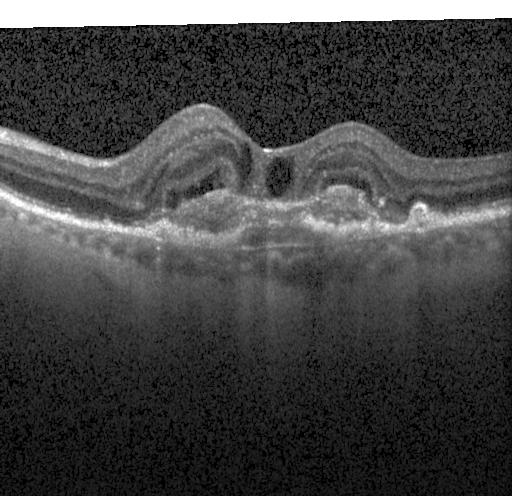

Assessment: CNV.